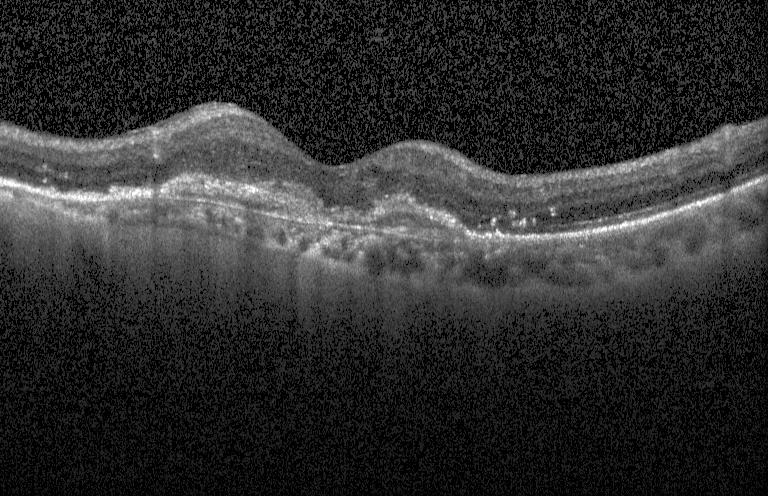

Optical coherence tomography scan · SD-OCT · instrument: Heidelberg Spectralis · centered on the fovea. The scan shows a choroidal neovascular membrane.